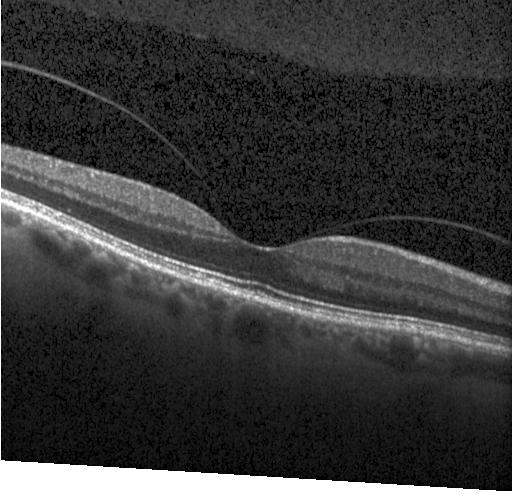 Diagnosis: no evidence of choroidal neovascularization, diabetic macular edema, or drusen.